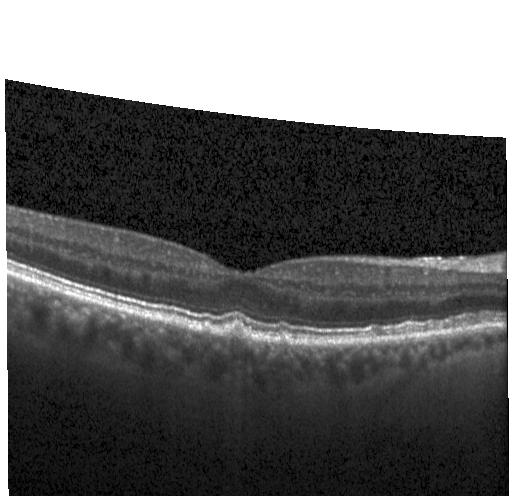 OCT B-scan showing multiple drusen.